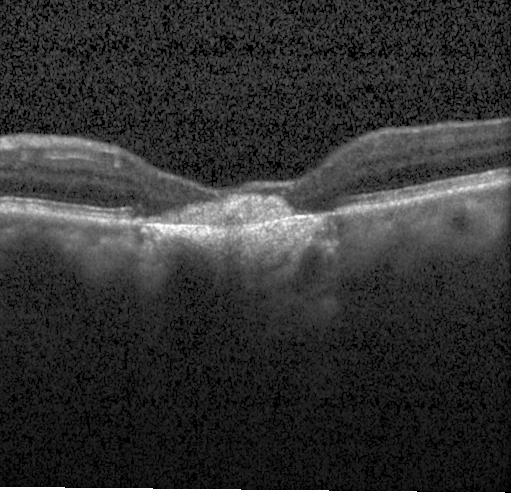

OCT B-scan showing CNV.